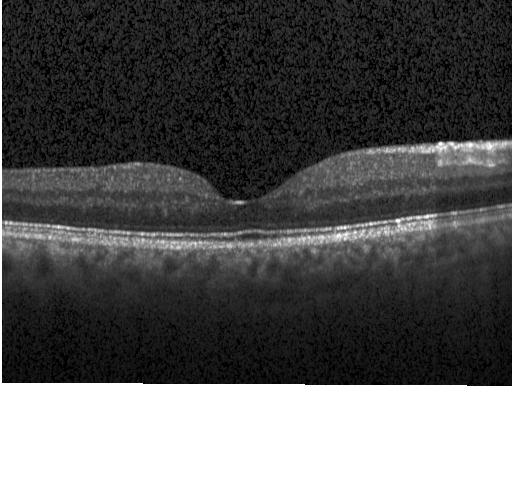
Finding: neither choroidal neovascularization, diabetic macular edema, nor drusen.